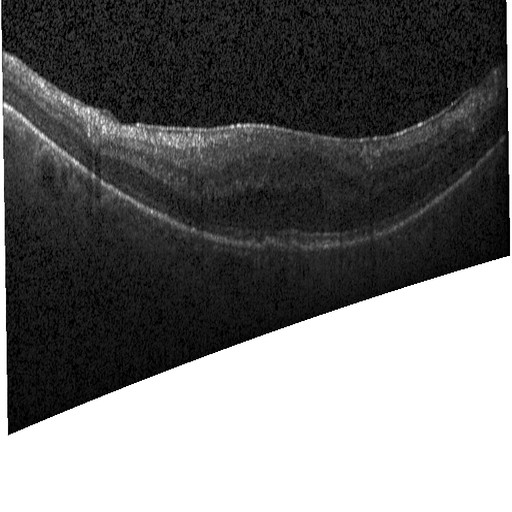 Acquired on a Heidelberg Spectralis; SD-OCT; OCT B-scan.
Finding: diabetic macular edema (DME).